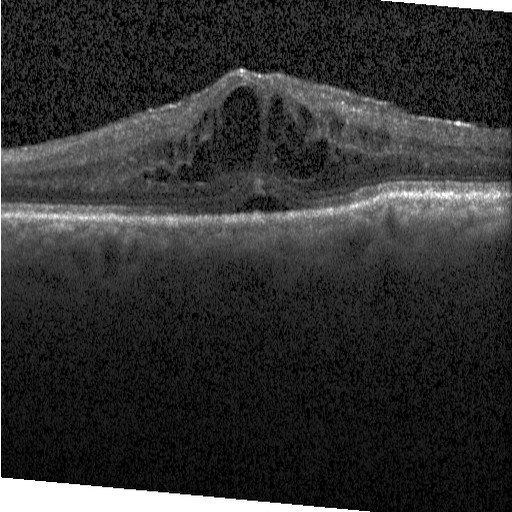 Fovea-centered; instrument: Heidelberg Spectralis; OCT B-scan; spectral-domain optical coherence tomography.
Impression: diabetic macular edema.